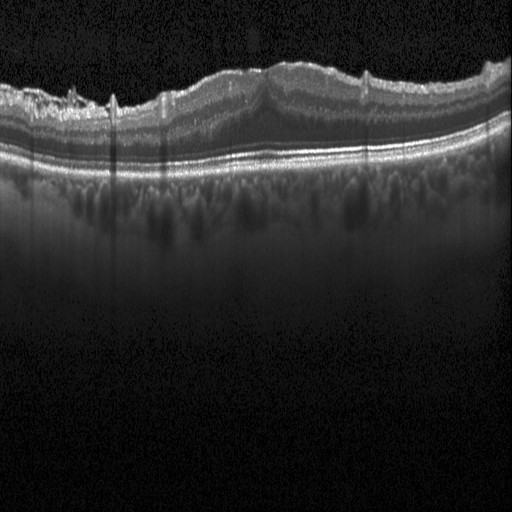

Macular OCT: DME.